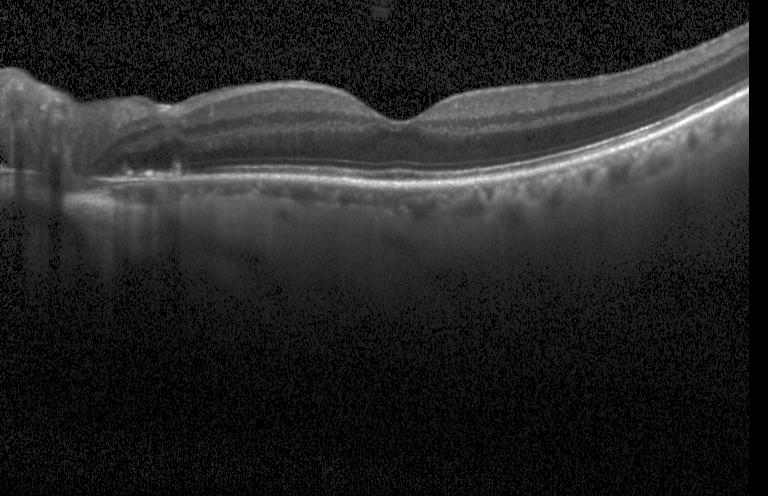

This B-scan demonstrates no CNV, DME, or drusen.